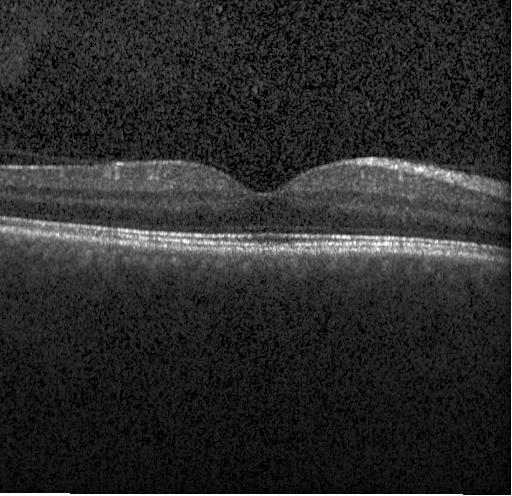

OCT B-scan
Impression: neither choroidal neovascularization, diabetic macular edema, nor drusen.